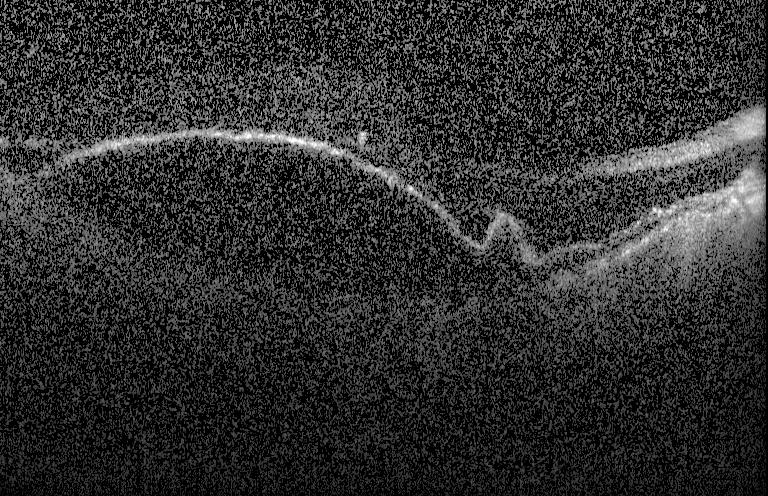 Centered on the fovea, retinal OCT cross-section
Assessment: choroidal neovascularization.